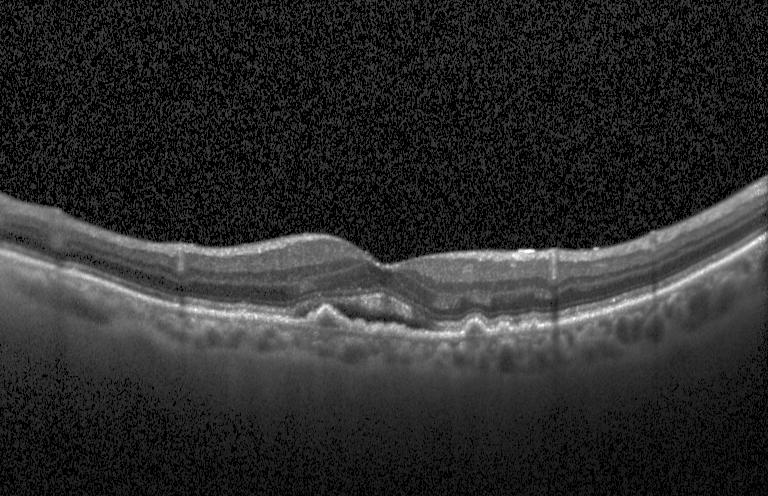 Through the macula. Retinal OCT B-scan. SD-OCT — A choroidal neovascular membrane.